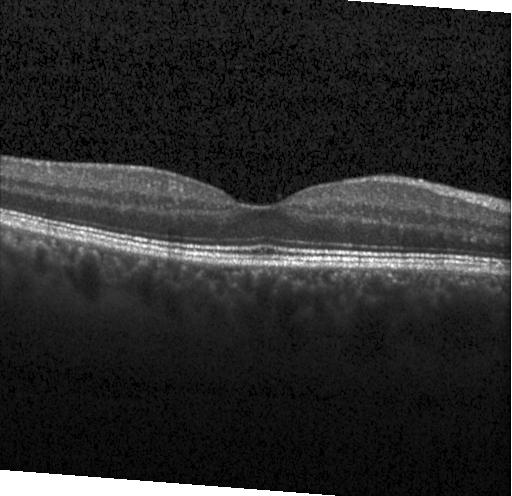
Optical coherence tomography B-scan; Heidelberg Spectralis; fovea-centered. Macular OCT: no choroidal neovascularization, no diabetic macular edema, and no drusen.